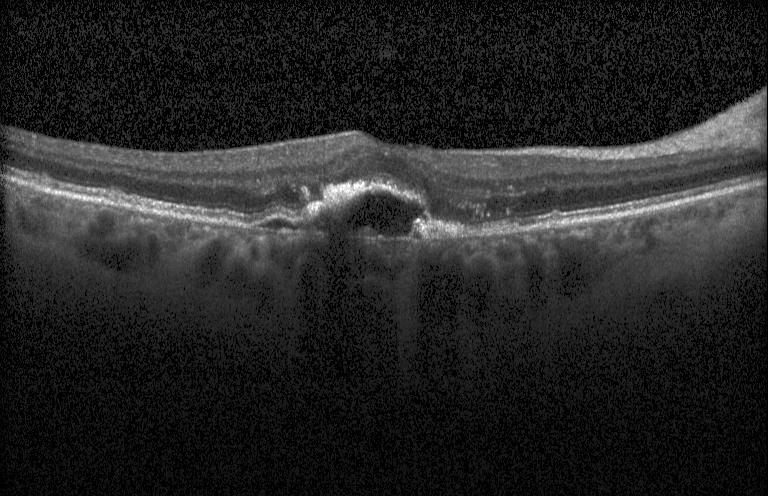

Centered on the fovea; retinal OCT cross-section; spectral-domain OCT — Macular OCT: choroidal neovascularization.